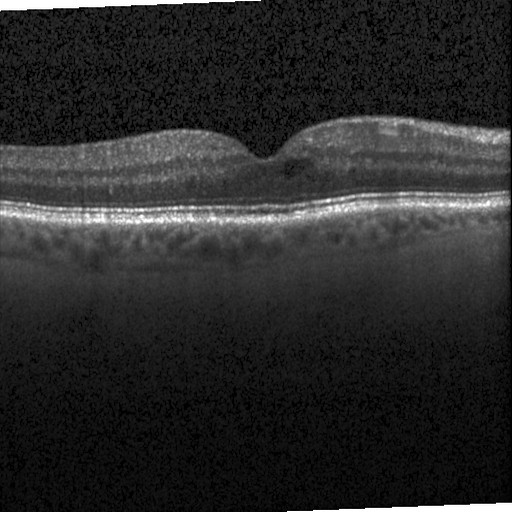

OCT scan showing diabetic macular edema.